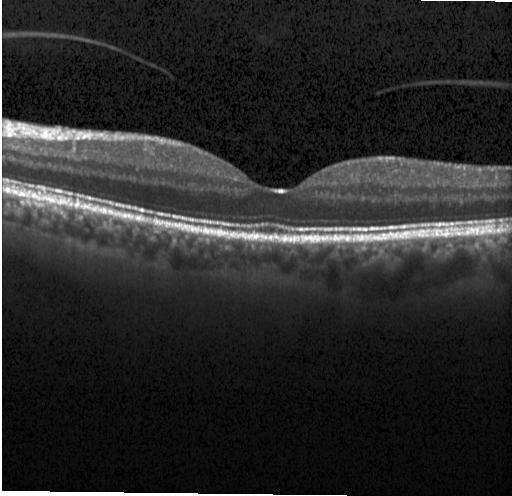

OCT line scan · instrument: Heidelberg Spectralis · through the macula · spectral-domain optical coherence tomography.
Dx: no choroidal neovascularization, no diabetic macular edema, and no drusen.